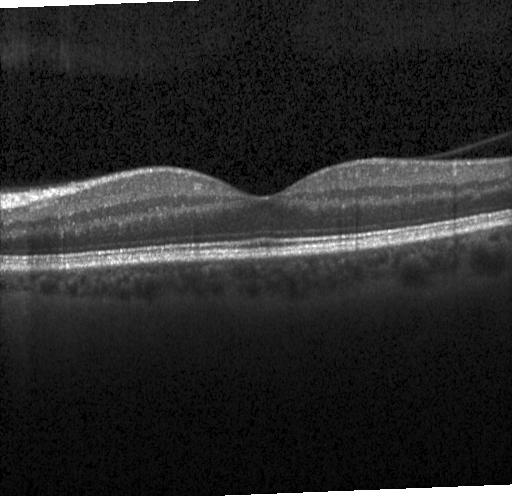 No evidence of choroidal neovascularization, diabetic macular edema, or drusen.